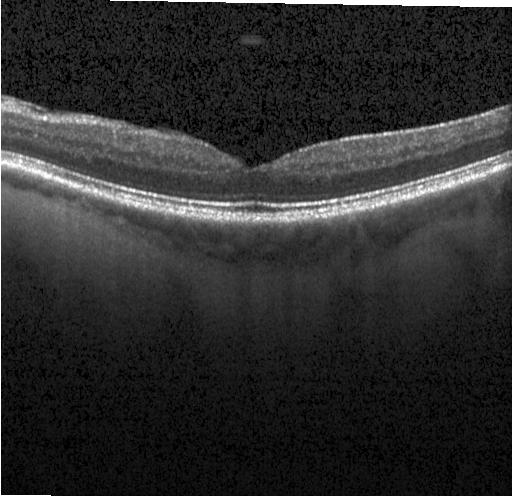
Retinal OCT cross-section showing no evidence of choroidal neovascularization, diabetic macular edema, or drusen.